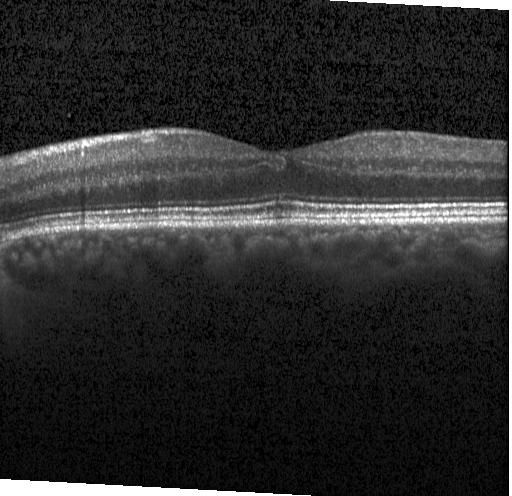 Fovea-centered, spectral-domain optical coherence tomography, retinal OCT B-scan — The scan shows no CNV, DME, or drusen.